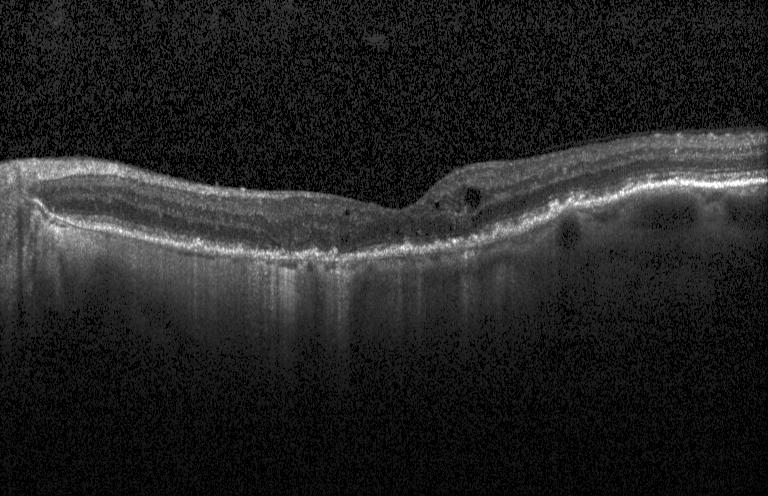
Finding: CNV.